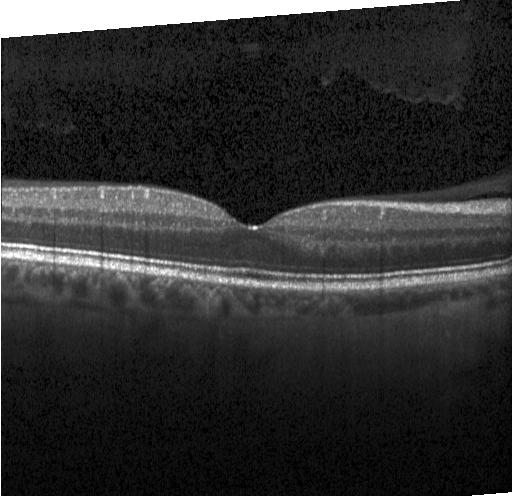 Retinal OCT B-scan. Dx: neither choroidal neovascularization, diabetic macular edema, nor drusen.